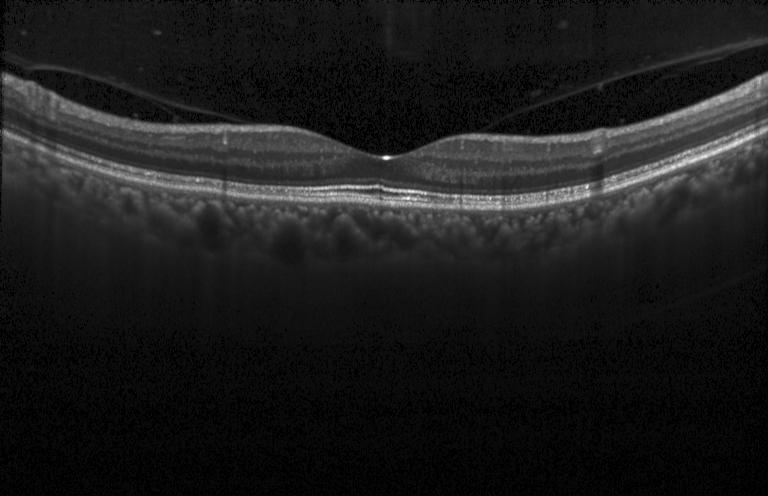

Centered on the fovea, retinal OCT B-scan, SD-OCT
The scan shows no choroidal neovascularization, diabetic macular edema, or drusen.